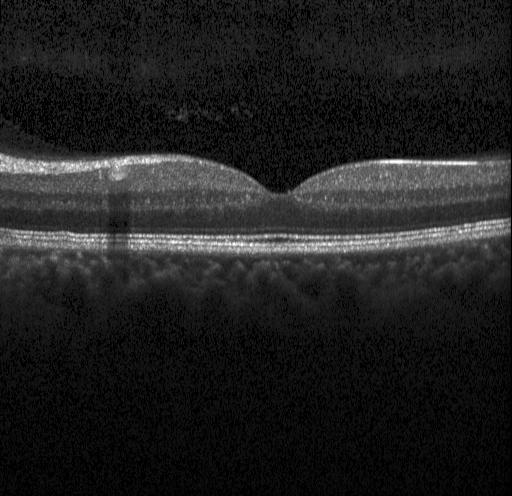
Macular OCT: neither choroidal neovascularization, diabetic macular edema, nor drusen.